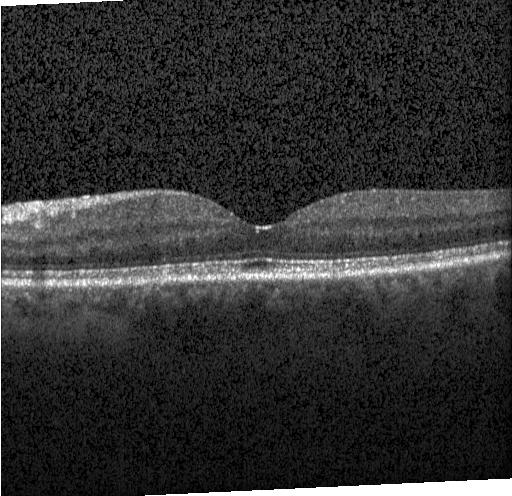 Macular scan. Retinal OCT cross-section.
The scan shows no evidence of choroidal neovascularization, diabetic macular edema, or drusen.